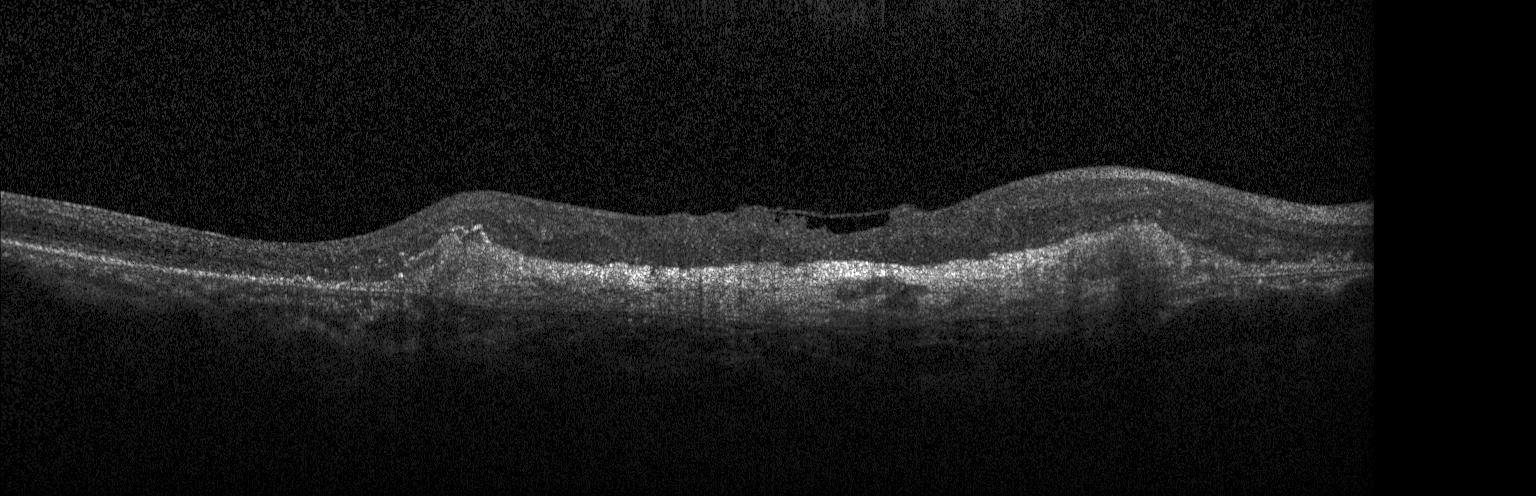 OCT line scan, spectral-domain optical coherence tomography — Finding: CNV.